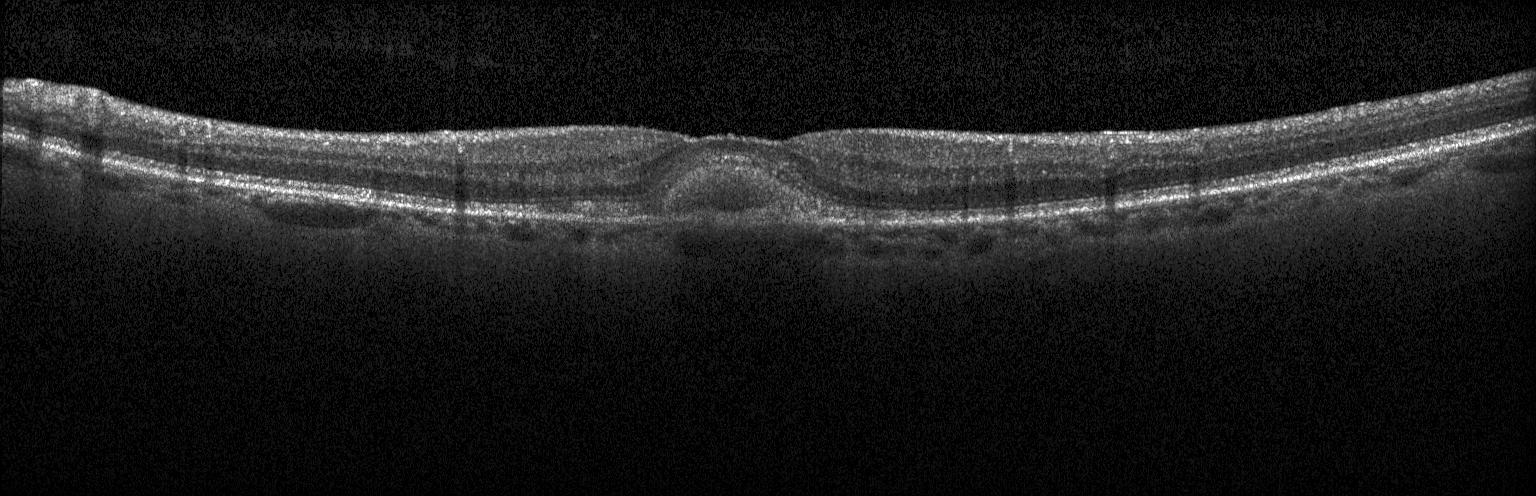
Retinal OCT cross-section; centered on the fovea; spectral-domain OCT — Impression: a choroidal neovascular membrane.